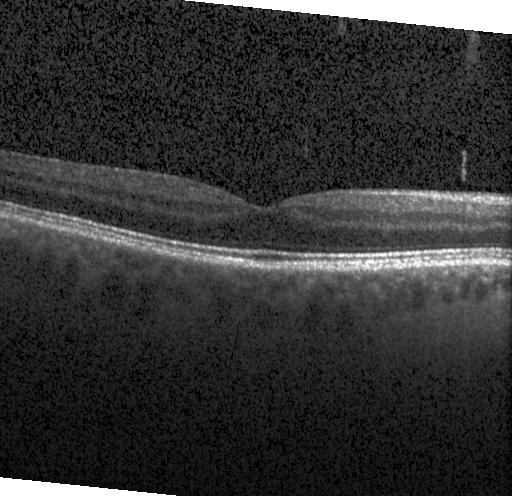

OCT finding: neither choroidal neovascularization, diabetic macular edema, nor drusen.